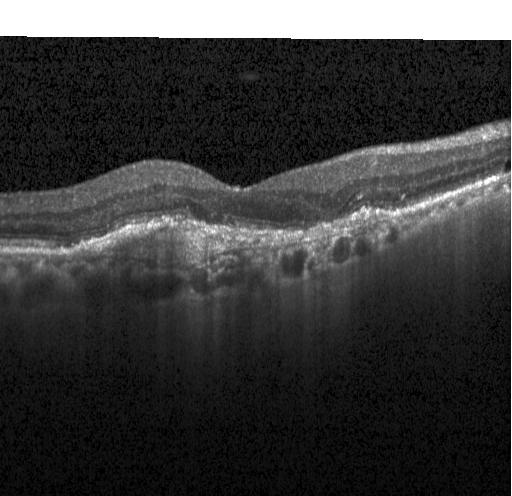 Instrument: Heidelberg Spectralis; horizontal scan through the fovea; optical coherence tomography B-scan — Finding: choroidal neovascularization.